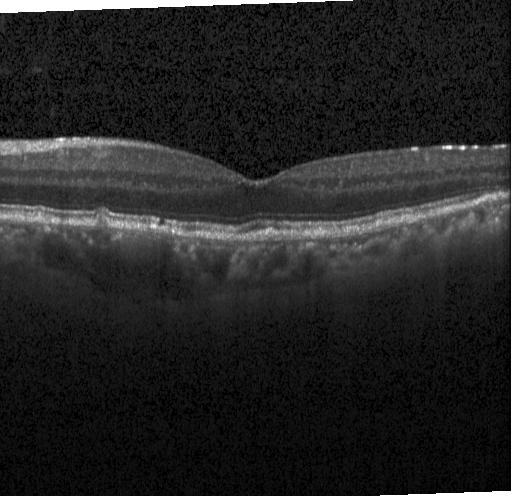 Optical coherence tomography scan · spectral-domain optical coherence tomography — Impression: drusen.